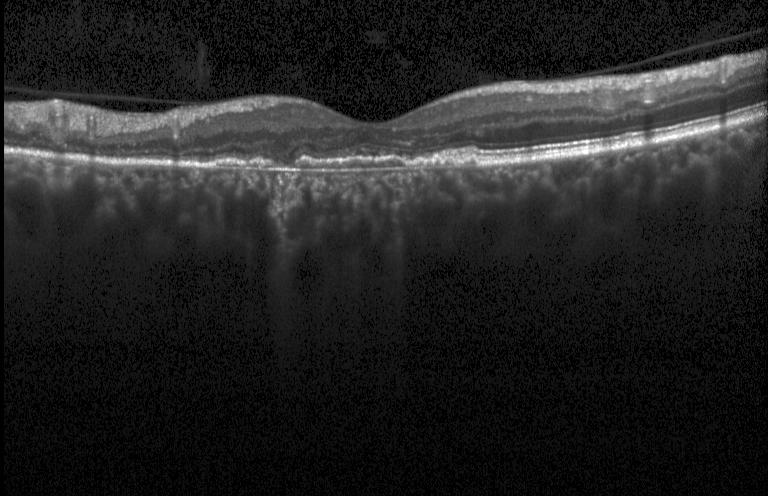
Diagnosis: a choroidal neovascular membrane.